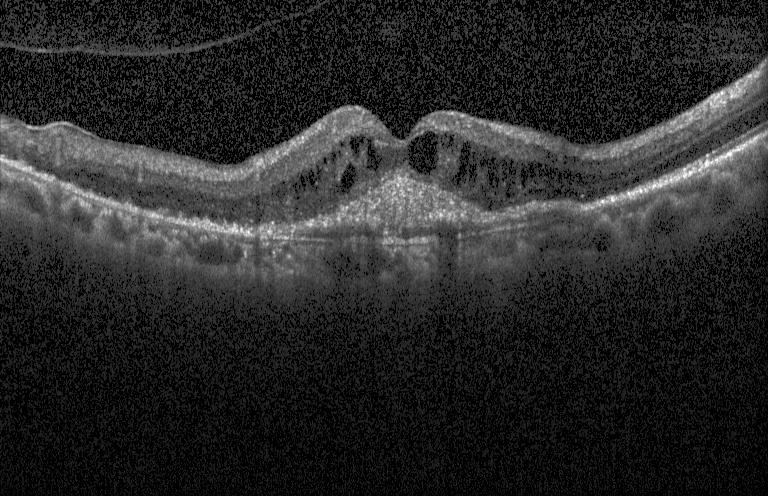

This B-scan demonstrates a choroidal neovascular membrane.